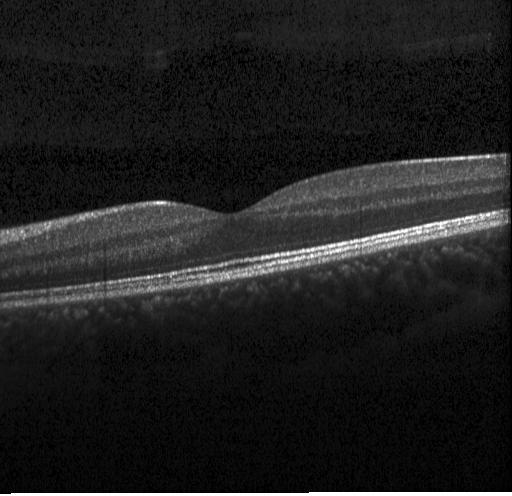

Retinal OCT B-scan. Impression: no choroidal neovascularization, no diabetic macular edema, and no drusen.